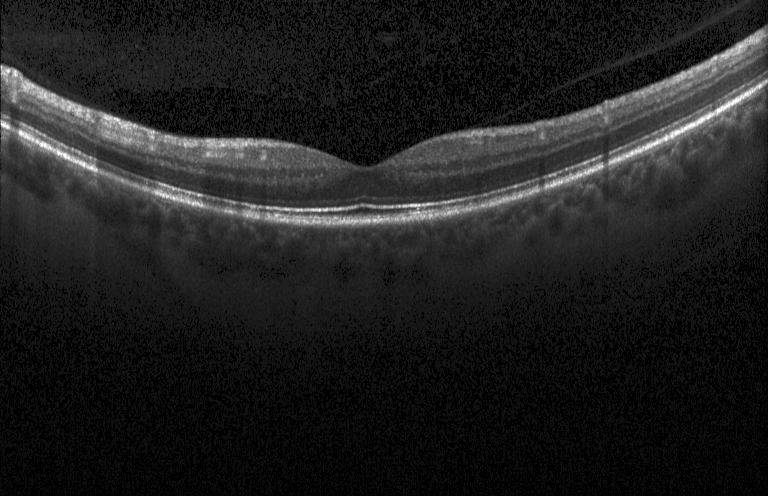 The scan shows neither choroidal neovascularization, diabetic macular edema, nor drusen.